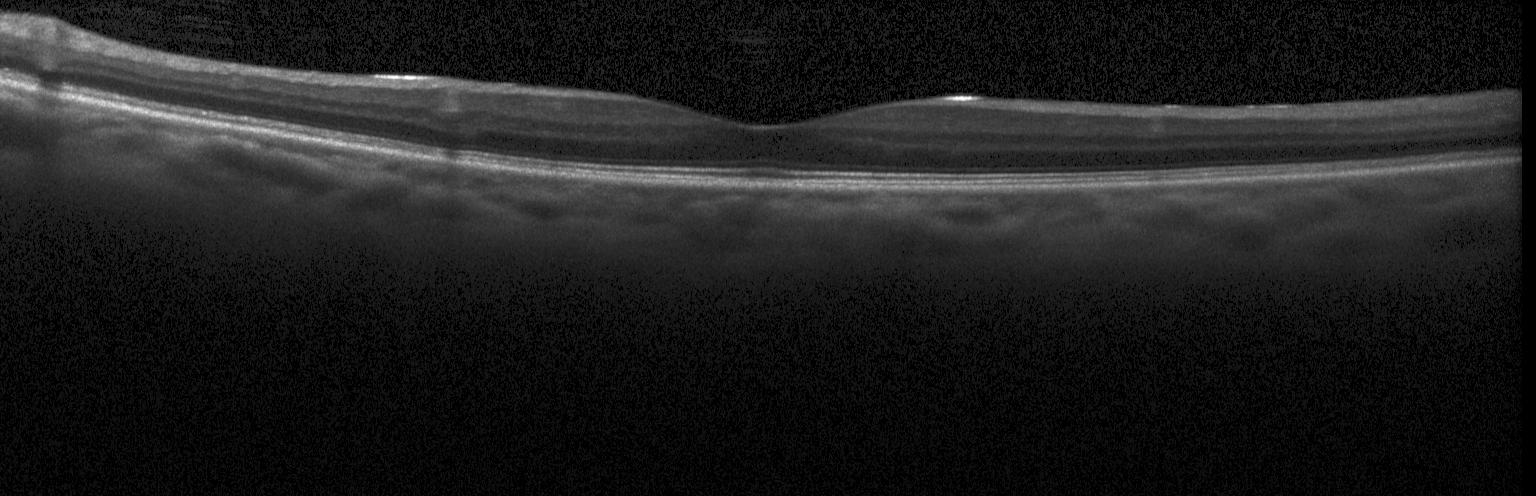
Through the macula, retinal OCT cross-section.
Diagnosis: neither choroidal neovascularization, diabetic macular edema, nor drusen.